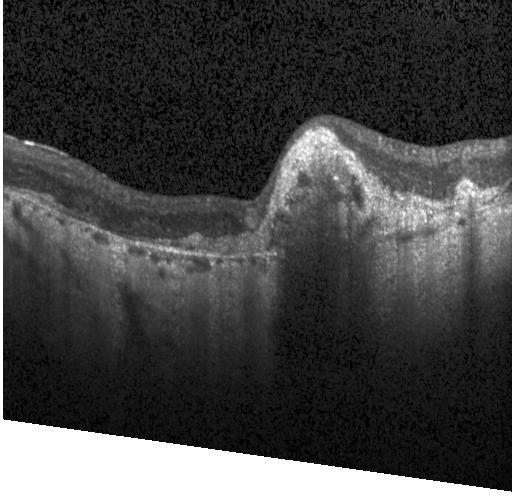

OCT finding: a choroidal neovascular membrane.